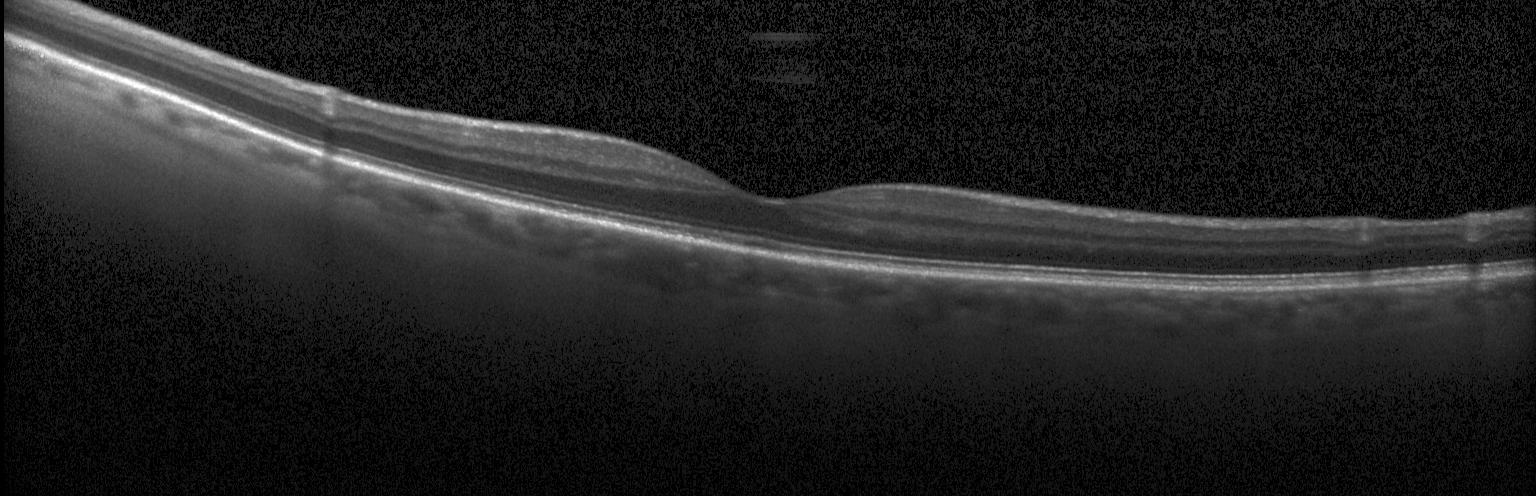 OCT scan showing neither choroidal neovascularization, diabetic macular edema, nor drusen.